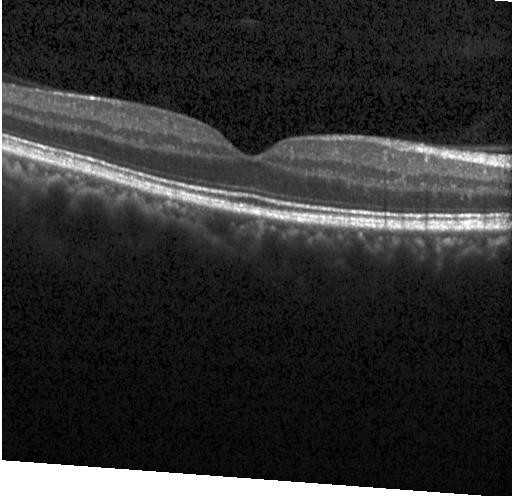
Retinal OCT B-scan
Finding: neither CNV, DME, nor drusen.